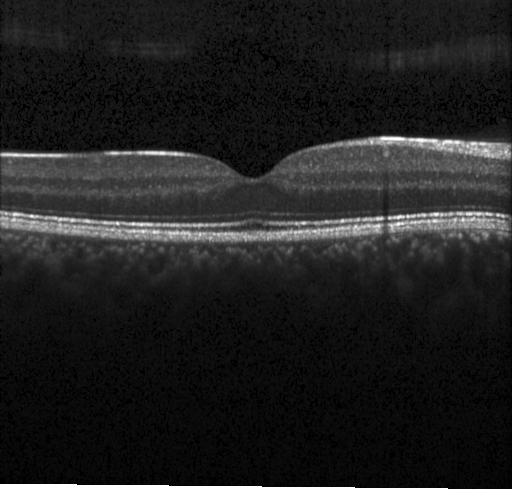

Optical coherence tomography scan. Diagnosis: no choroidal neovascularization, no diabetic macular edema, and no drusen.